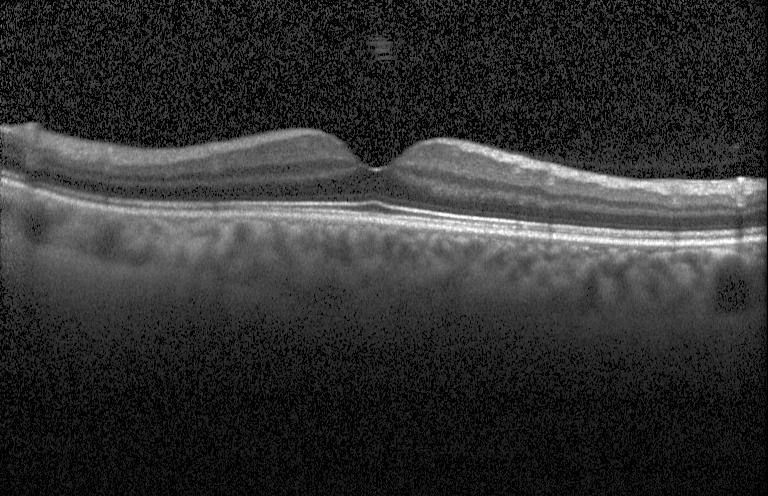
Centered on the fovea, instrument: Heidelberg Spectralis, spectral-domain optical coherence tomography, optical coherence tomography B-scan. Finding: no CNV, no DME, and no drusen.